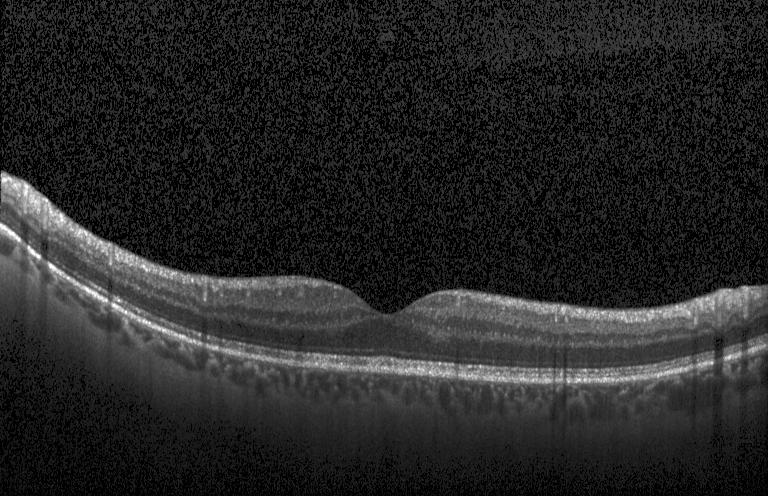
Impression: no choroidal neovascularization, no diabetic macular edema, and no drusen.